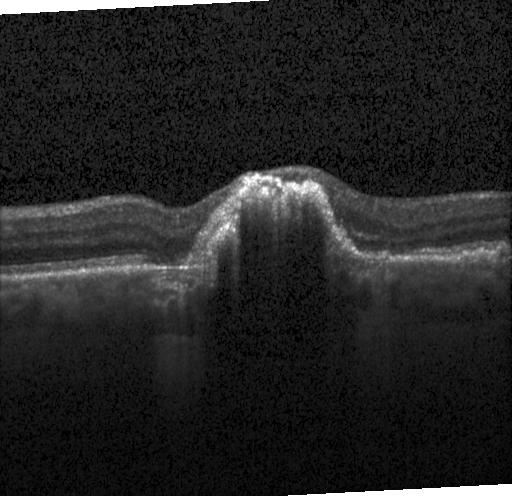

Finding: choroidal neovascularization (CNV).